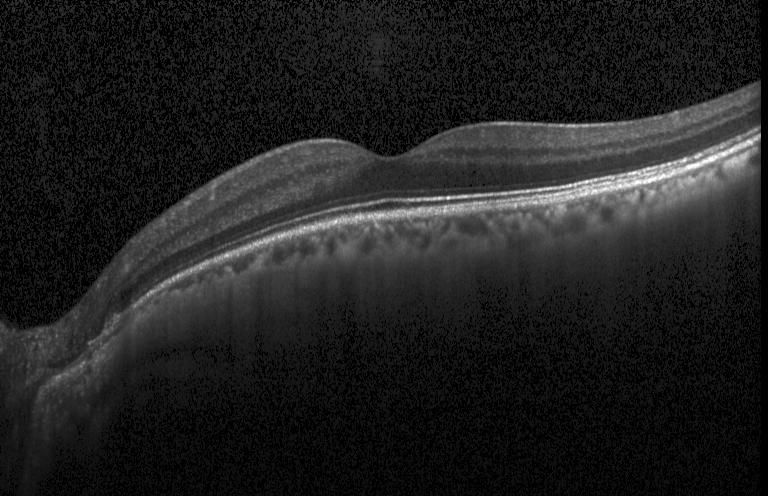
SD-OCT. Instrument: Heidelberg Spectralis. Macular scan. OCT B-scan. Impression: neither choroidal neovascularization, diabetic macular edema, nor drusen.